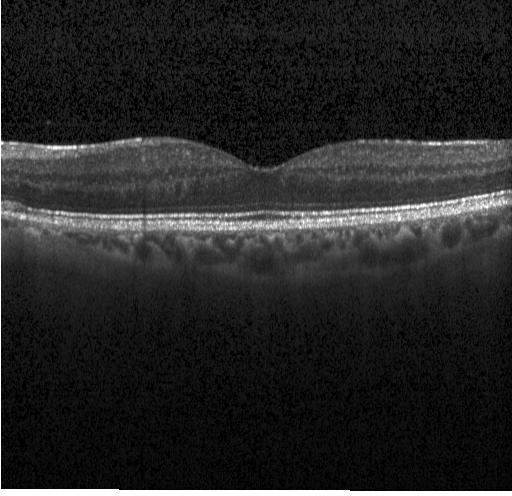 Impression: no evidence of CNV, DME, or drusen.